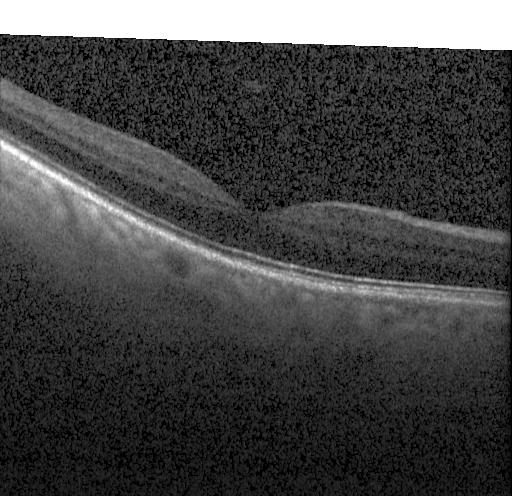 Macular OCT: neither choroidal neovascularization, diabetic macular edema, nor drusen.